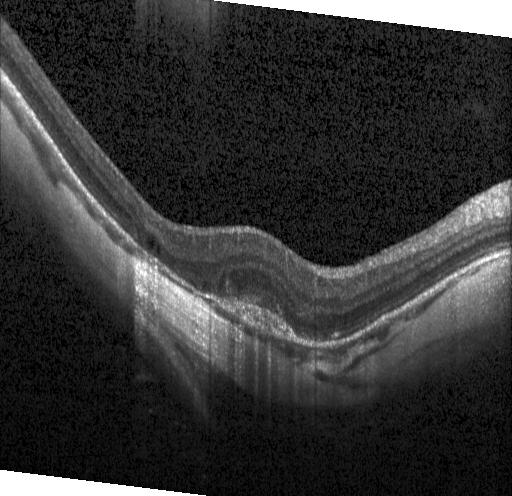

Diagnosis: a choroidal neovascular membrane.